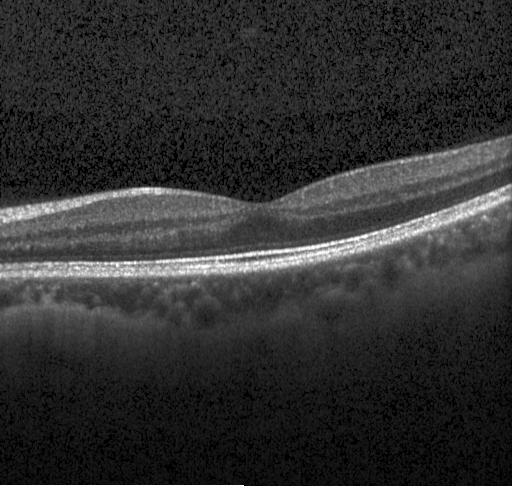 Instrument: Heidelberg Spectralis. Optical coherence tomography B-scan. The scan shows neither choroidal neovascularization, diabetic macular edema, nor drusen.